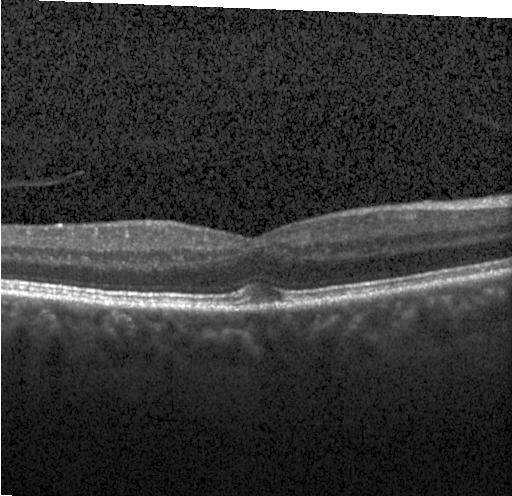

OCT finding: drusen.